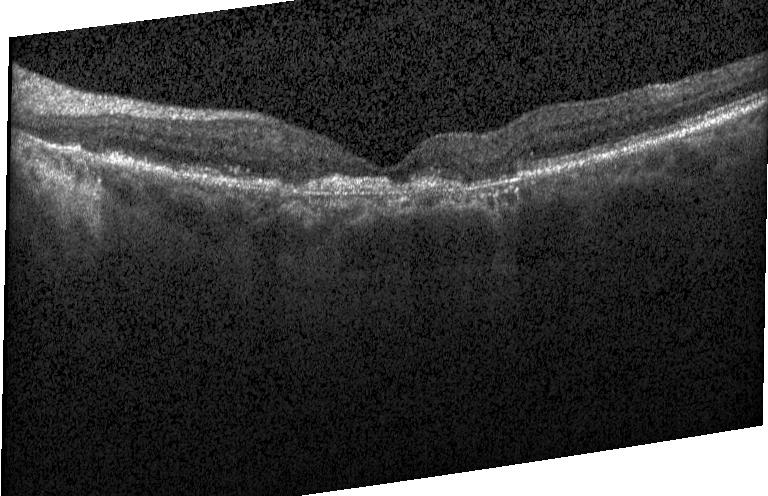
Dx: choroidal neovascularization (CNV).